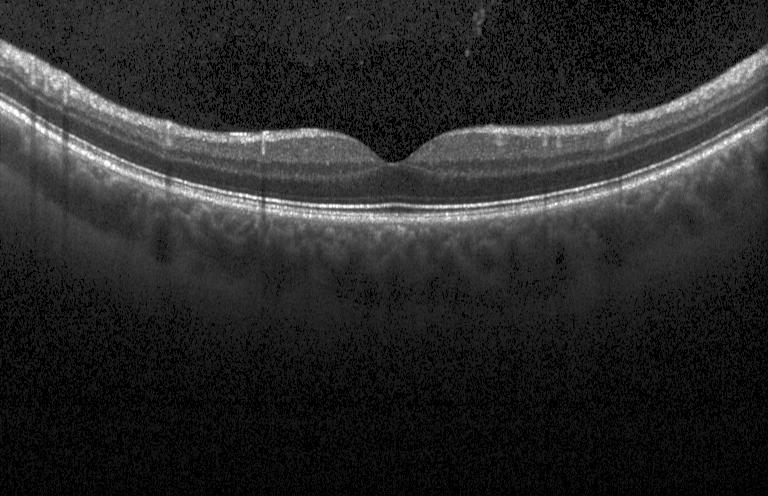
OCT line scan, spectral-domain OCT, acquired on a Heidelberg Spectralis, horizontal scan through the fovea — This B-scan demonstrates no CNV, no DME, and no drusen.